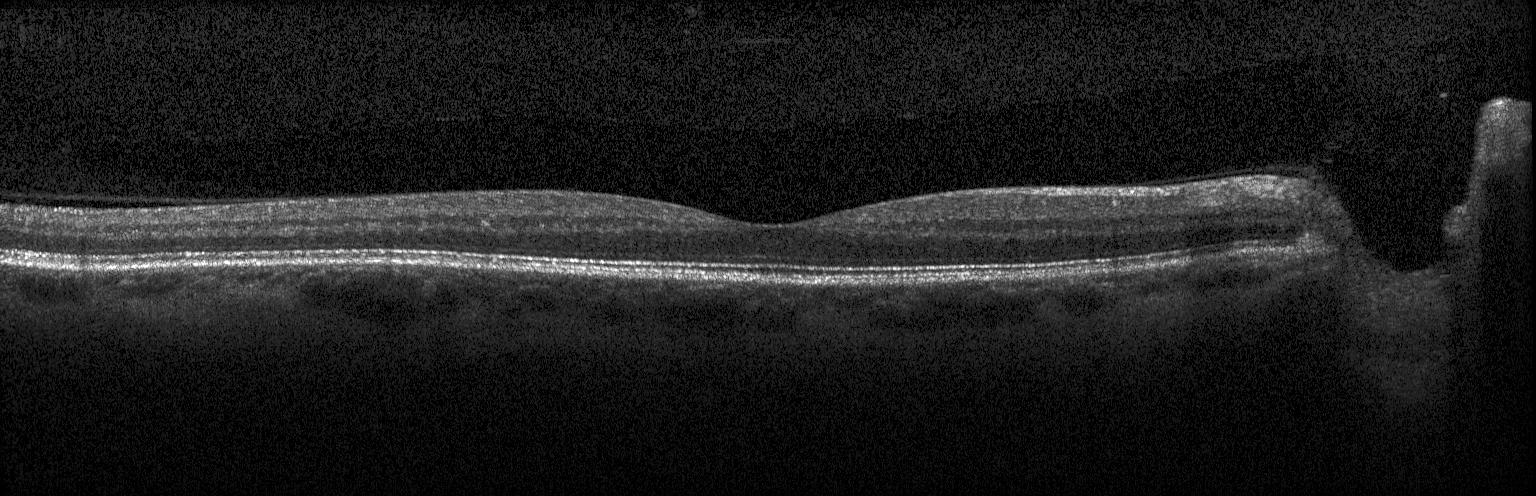 Retinal OCT B-scan.
Diagnosis: no evidence of CNV, DME, or drusen.